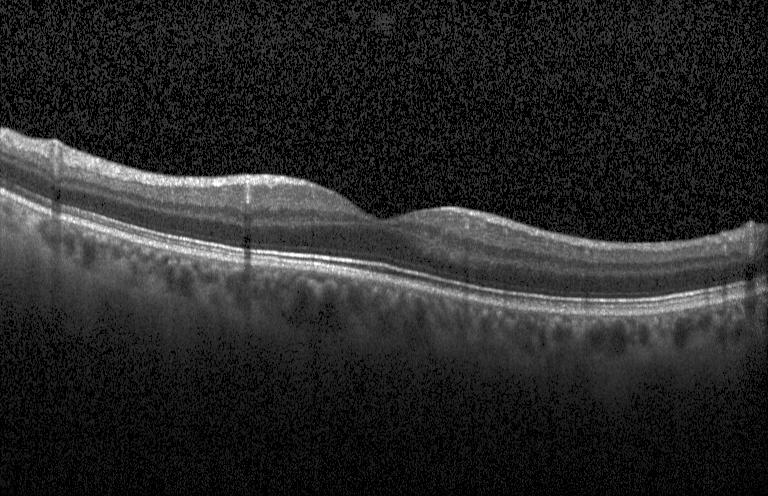 Assessment: neither choroidal neovascularization, diabetic macular edema, nor drusen.